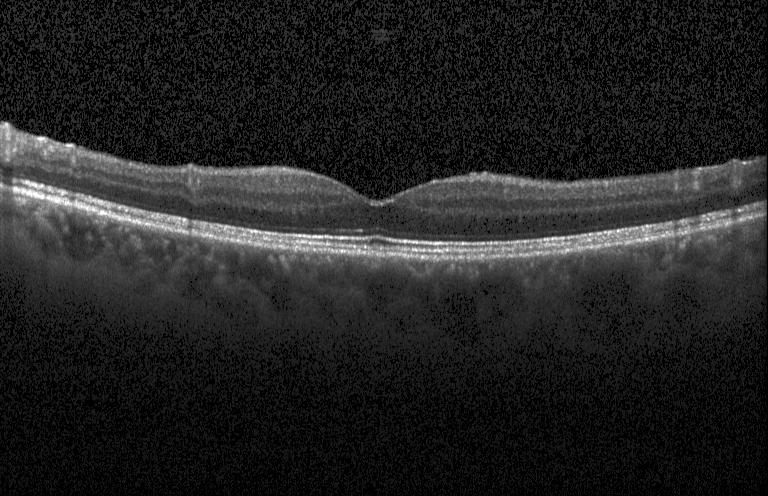 OCT finding: no CNV, DME, or drusen.